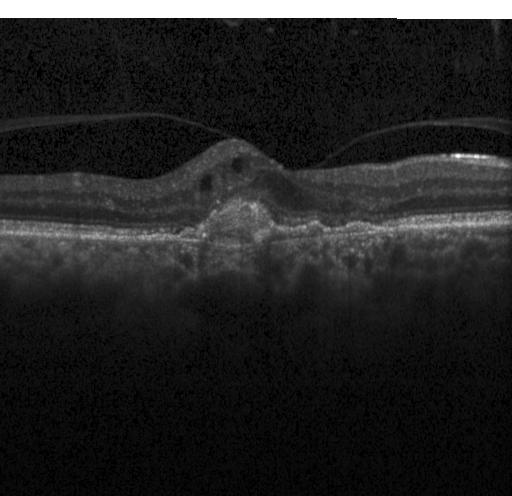 OCT B-scan showing choroidal neovascularization.